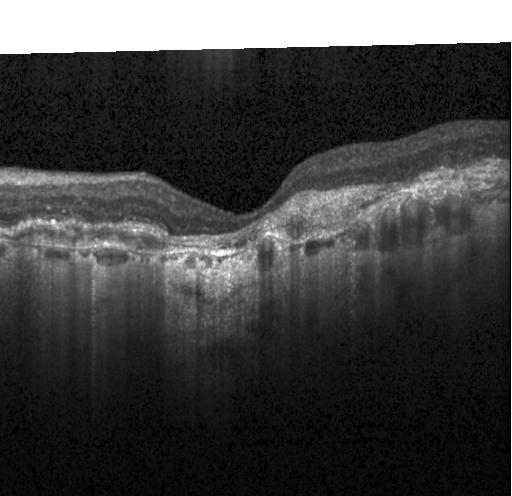
Macular OCT demonstrating a choroidal neovascular membrane.